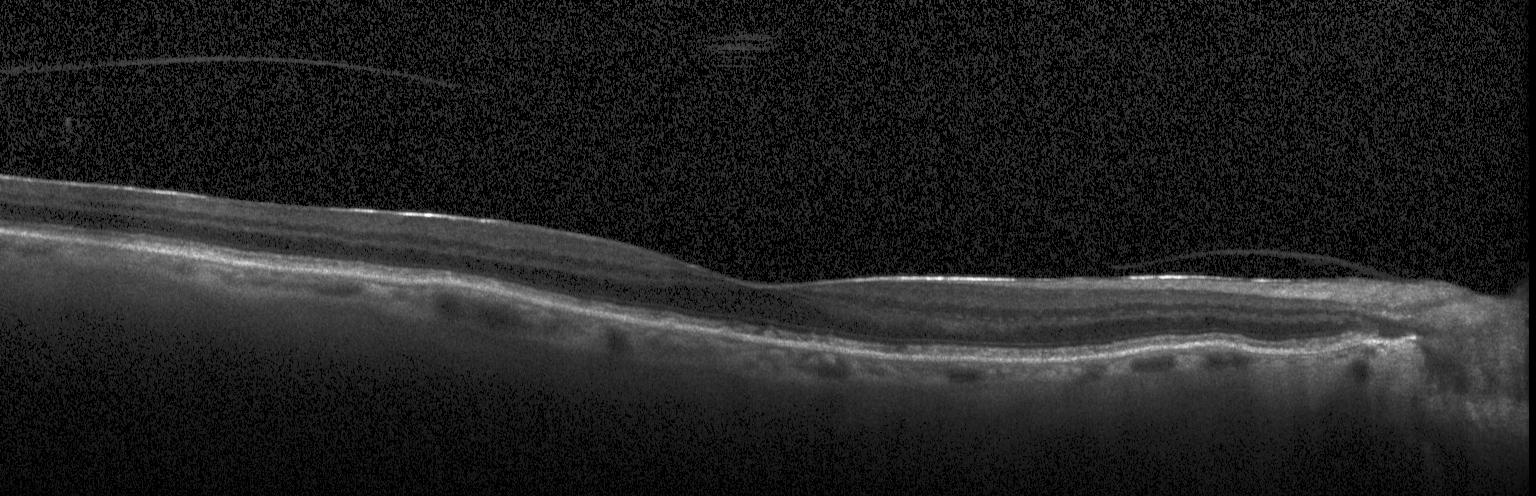 Through the macula, OCT B-scan, instrument: Heidelberg Spectralis, spectral-domain optical coherence tomography. This B-scan demonstrates no choroidal neovascularization, diabetic macular edema, or drusen.